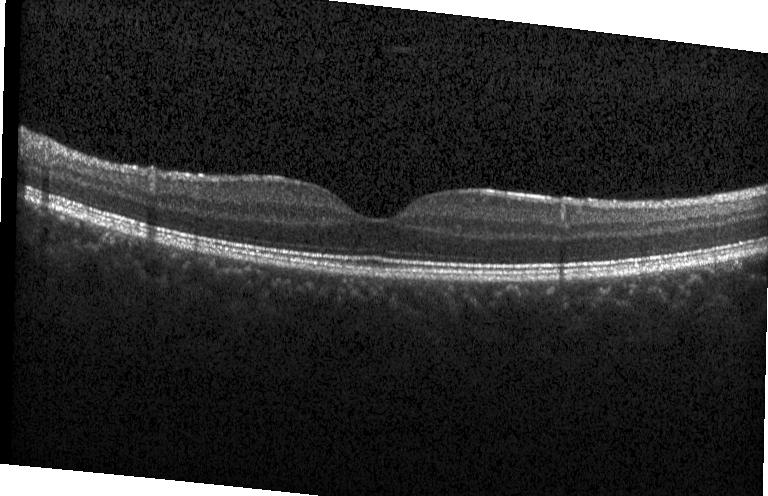
This B-scan demonstrates no choroidal neovascularization, diabetic macular edema, or drusen.